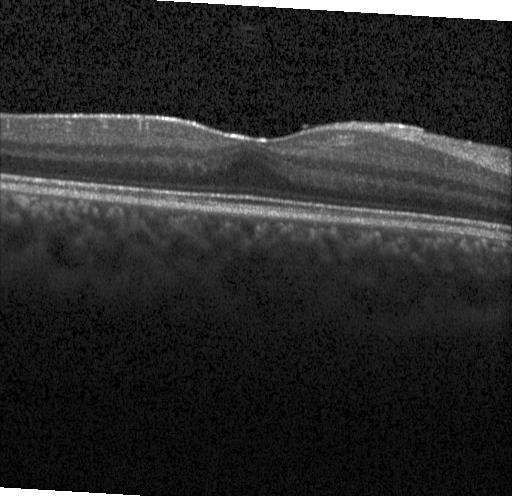

OCT B-scan.
No choroidal neovascularization, no diabetic macular edema, and no drusen.